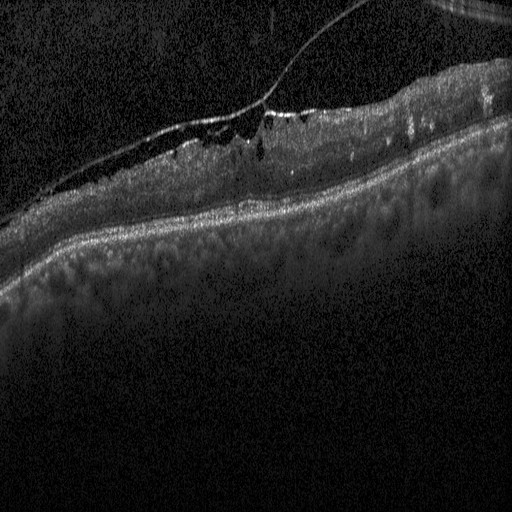
Diagnosis: DME.